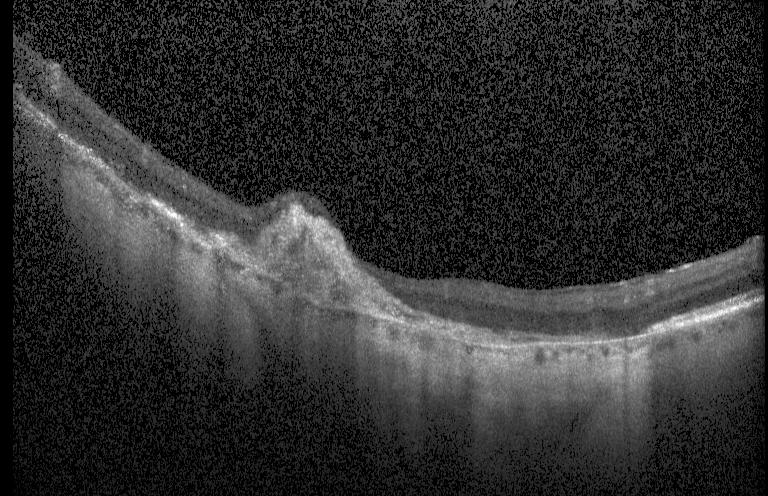 Optical coherence tomography scan · SD-OCT
OCT finding: a choroidal neovascular membrane.